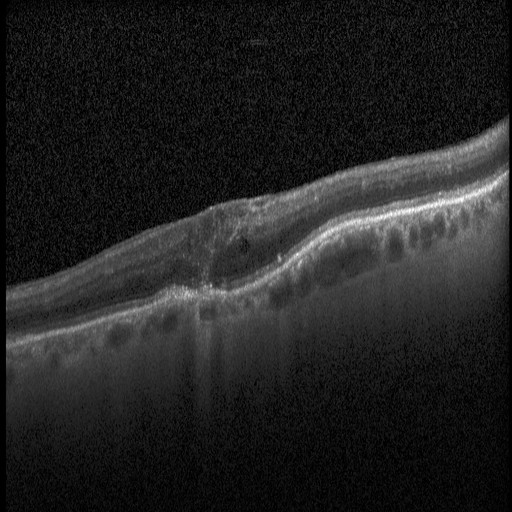
Optical coherence tomography B-scan — Diagnosis: DME.